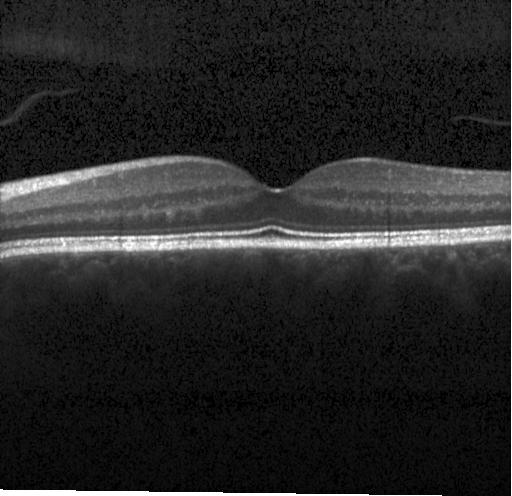
Dx: no choroidal neovascularization, no diabetic macular edema, and no drusen.